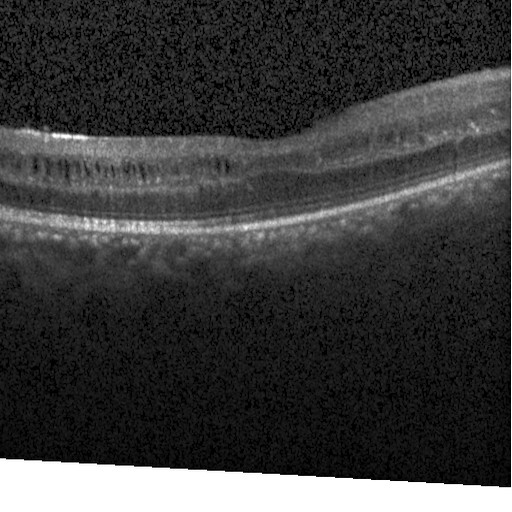

Heidelberg Spectralis · optical coherence tomography scan · SD-OCT.
Impression: diabetic macular edema.